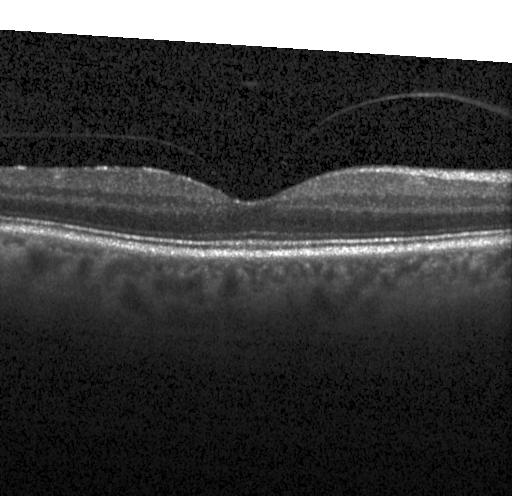 Heidelberg Spectralis OCT system · OCT line scan · through the macula
The scan shows no evidence of CNV, DME, or drusen.